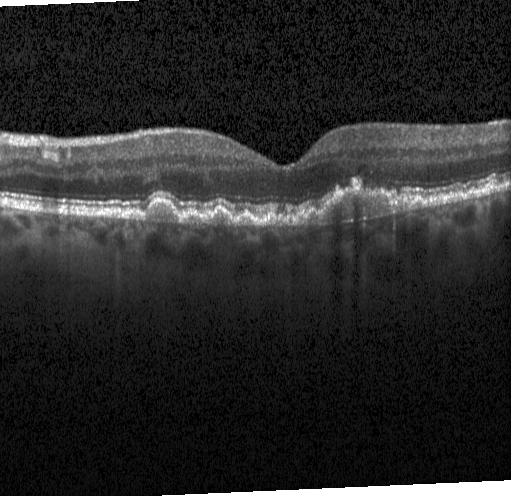
Spectral-domain OCT, optical coherence tomography B-scan, instrument: Heidelberg Spectralis. OCT finding: multiple drusen.